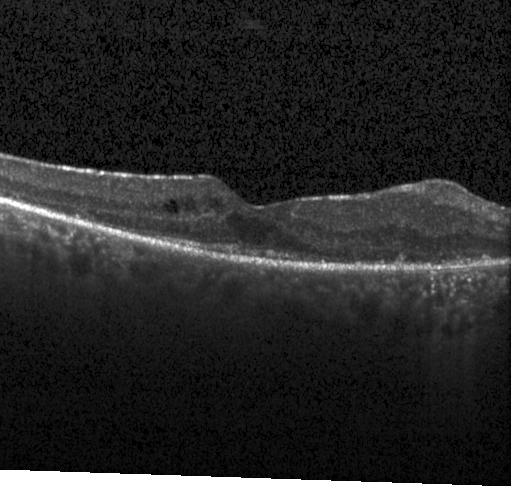
Retinal OCT cross-section showing diabetic macular edema.